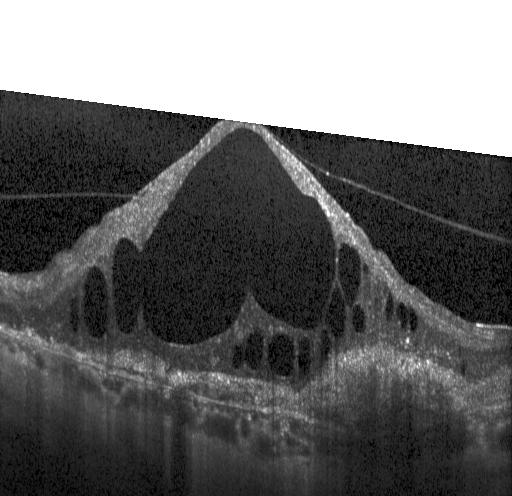 Impression: a choroidal neovascular membrane.